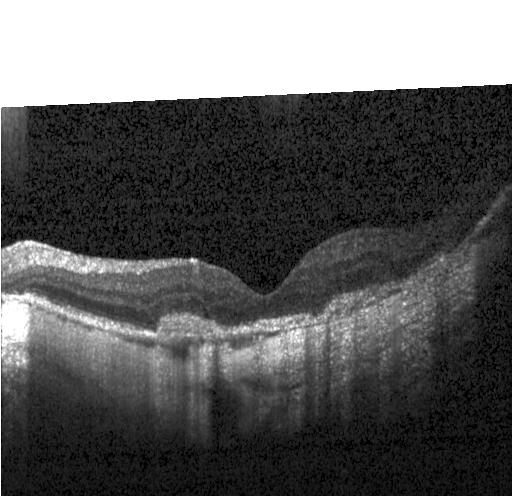
Optical coherence tomography scan.
This B-scan demonstrates CNV.